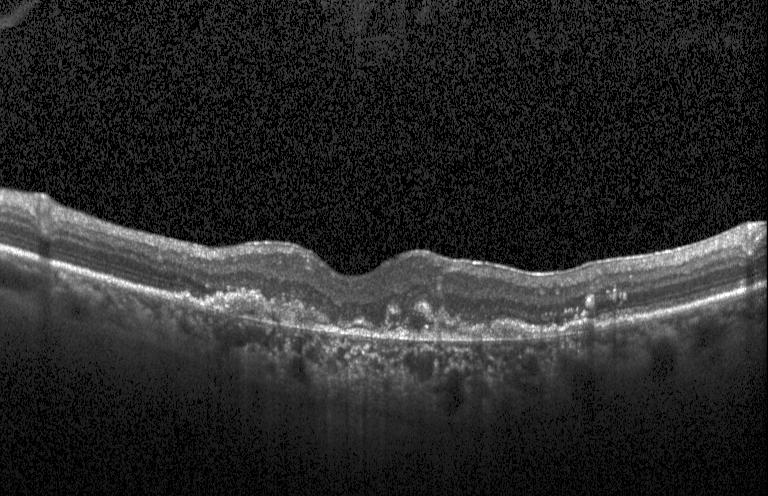 OCT B-scan showing choroidal neovascularization.